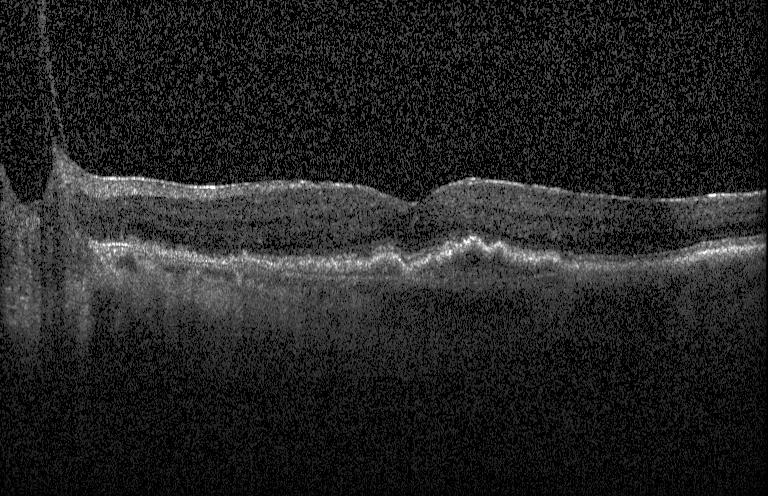
Centered on the fovea; instrument: Heidelberg Spectralis; optical coherence tomography B-scan. Diagnosis: choroidal neovascularization.